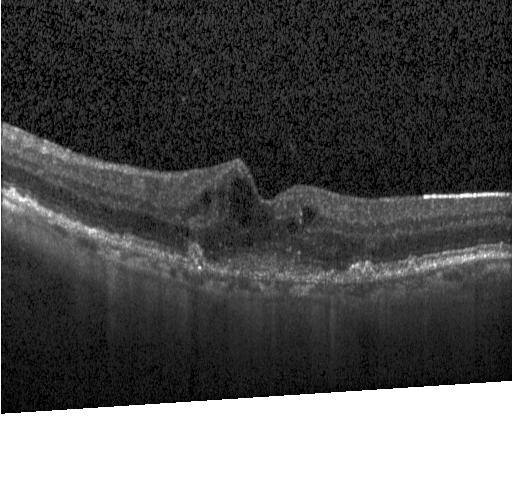 Optical coherence tomography scan. OCT finding: a choroidal neovascular membrane.